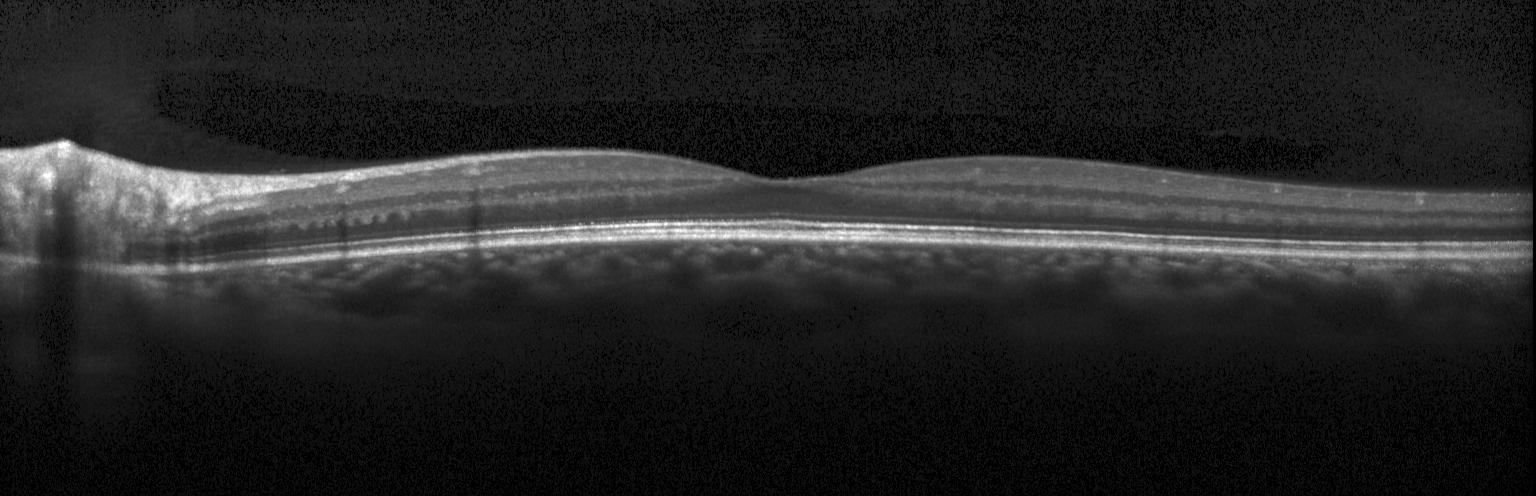
Retinal OCT B-scan, spectral-domain optical coherence tomography, centered on the fovea, acquired on a Heidelberg Spectralis
OCT finding: neither choroidal neovascularization, diabetic macular edema, nor drusen.